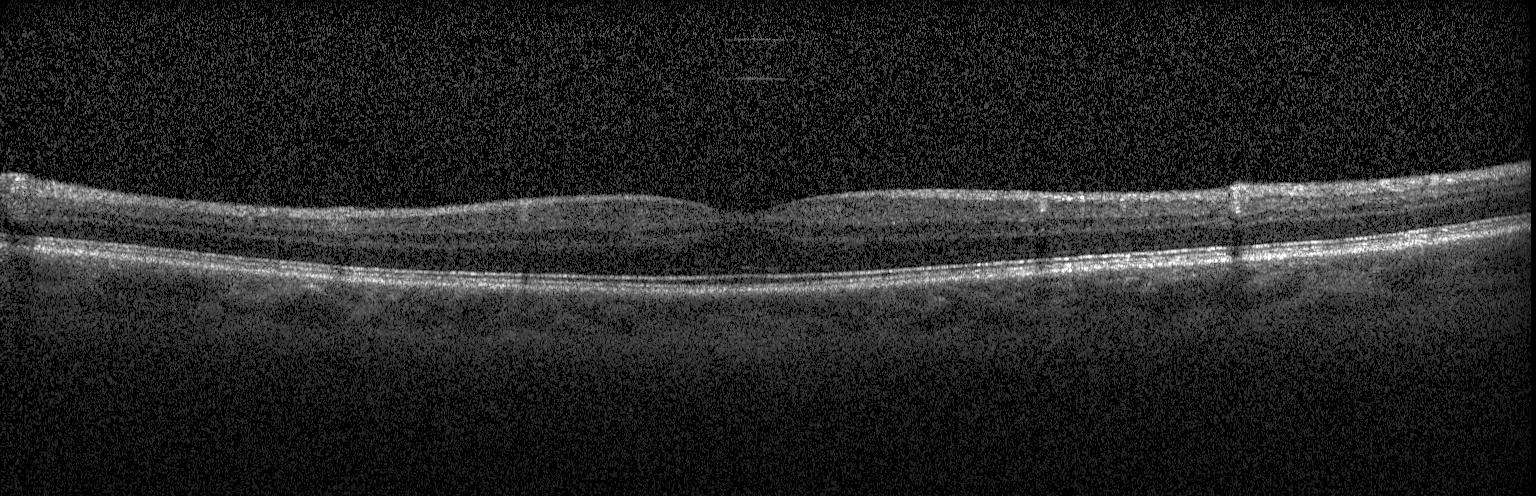 Finding: neither CNV, DME, nor drusen.